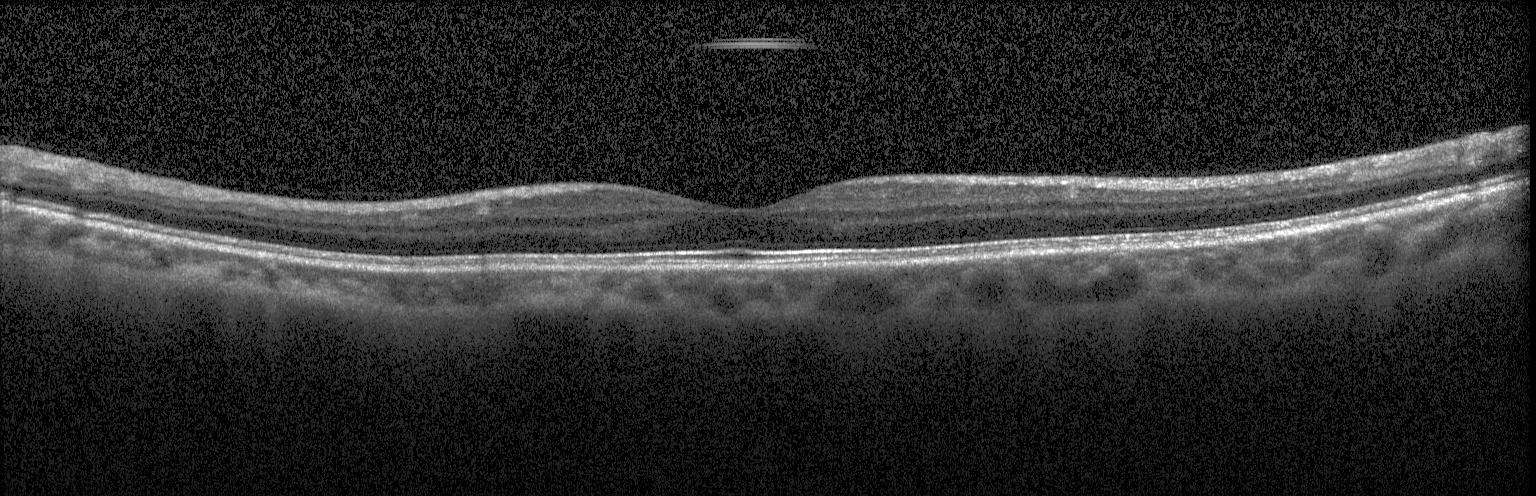 OCT finding: no choroidal neovascularization, no diabetic macular edema, and no drusen.